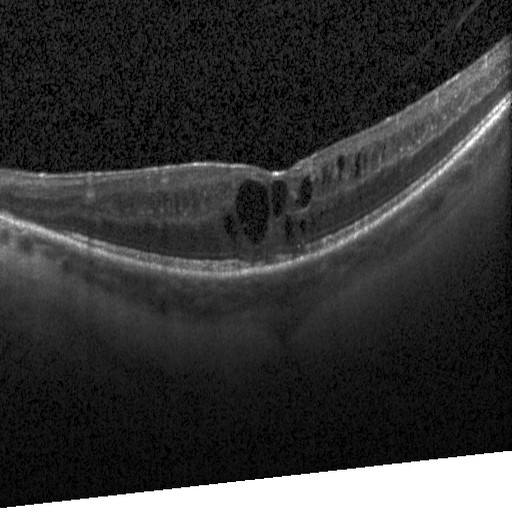
Diagnosis: DME.